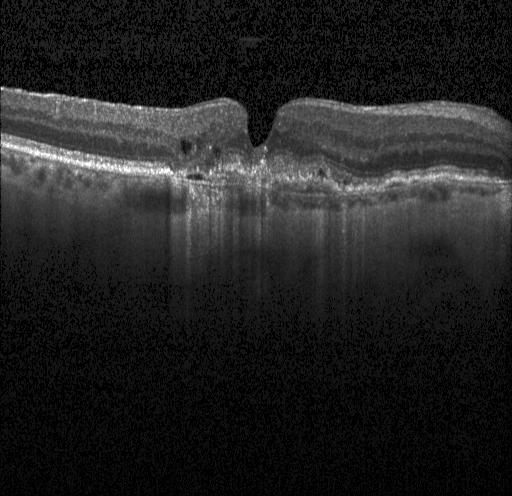
Retinal OCT cross-section; through the macula; Heidelberg Spectralis OCT system; SD-OCT.
Impression: a choroidal neovascular membrane.